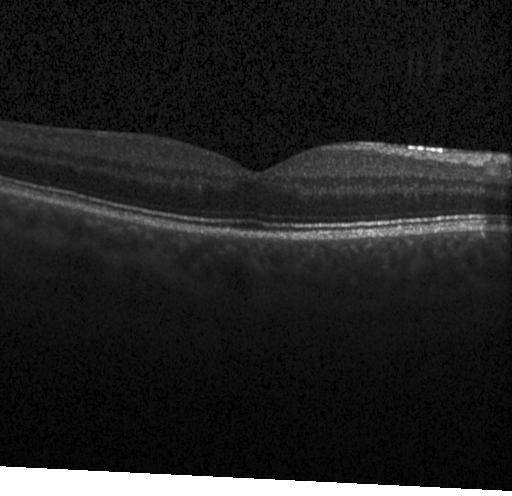 This B-scan demonstrates neither choroidal neovascularization, diabetic macular edema, nor drusen.